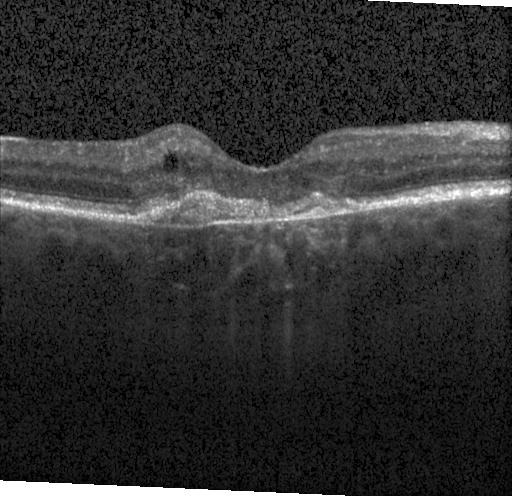
OCT line scan; spectral-domain optical coherence tomography
Dx: choroidal neovascularization (CNV).